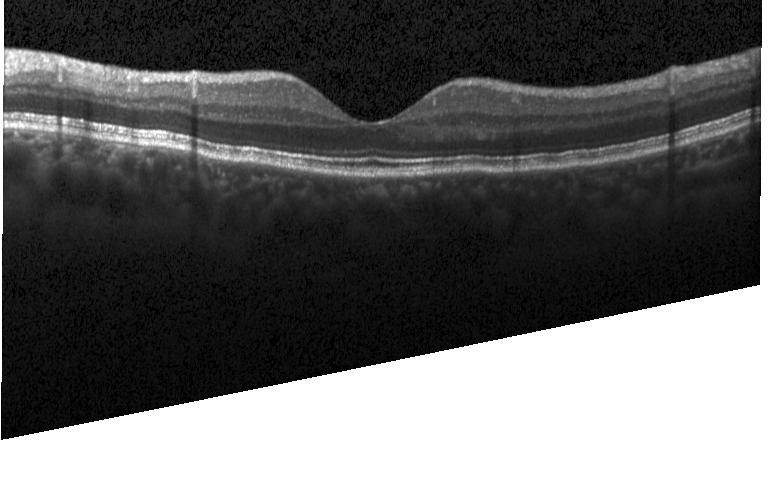 Retinal OCT B-scan. Finding: neither choroidal neovascularization, diabetic macular edema, nor drusen.